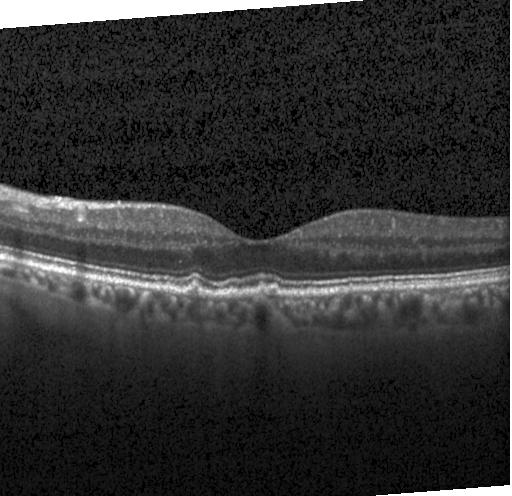
Centered on the fovea; retinal OCT cross-section. Dx: multiple drusen.